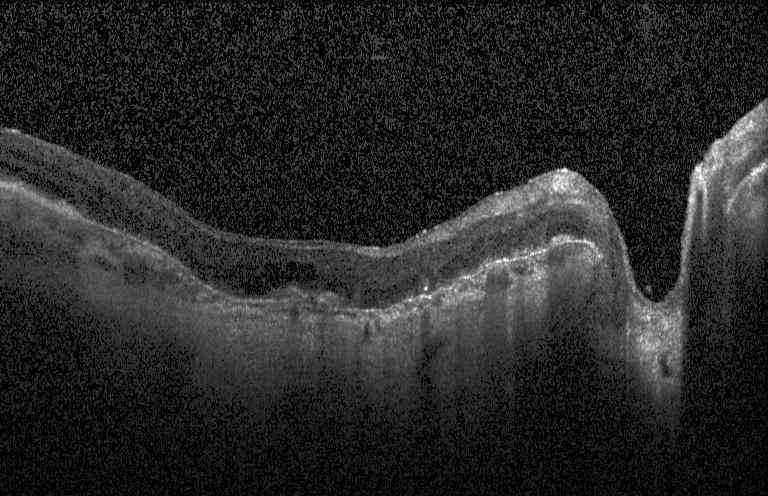
OCT line scan, instrument: Heidelberg Spectralis, spectral-domain OCT. Assessment: CNV.